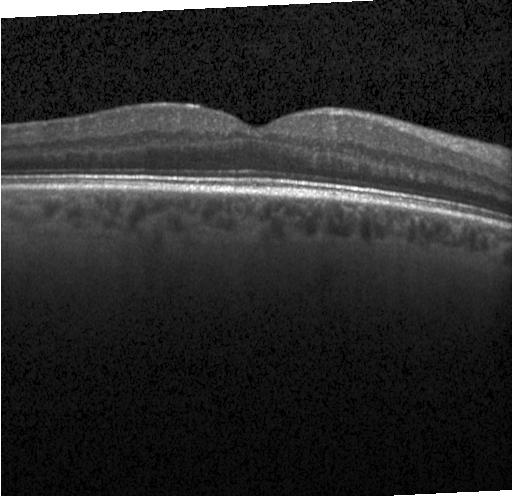 Finding: no choroidal neovascularization, diabetic macular edema, or drusen.